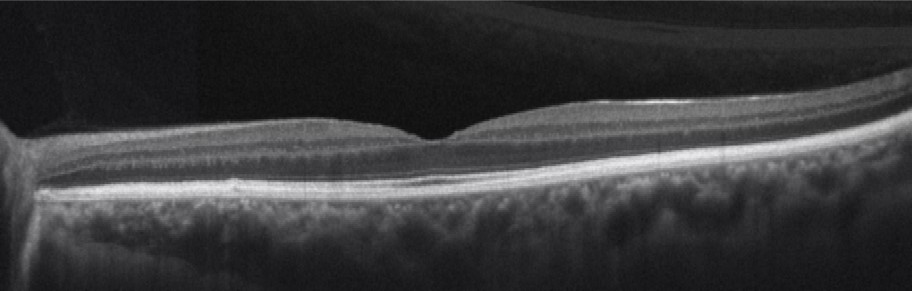
Macular OCT: no evidence of AMD, DME, ERM, RAO, RVO, or VID.